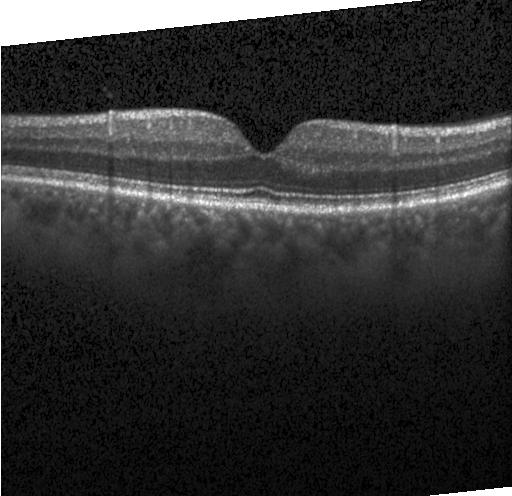 Spectral-domain optical coherence tomography. Heidelberg Spectralis OCT system. Optical coherence tomography B-scan. Fovea-centered.
Dx: no CNV, no DME, and no drusen.